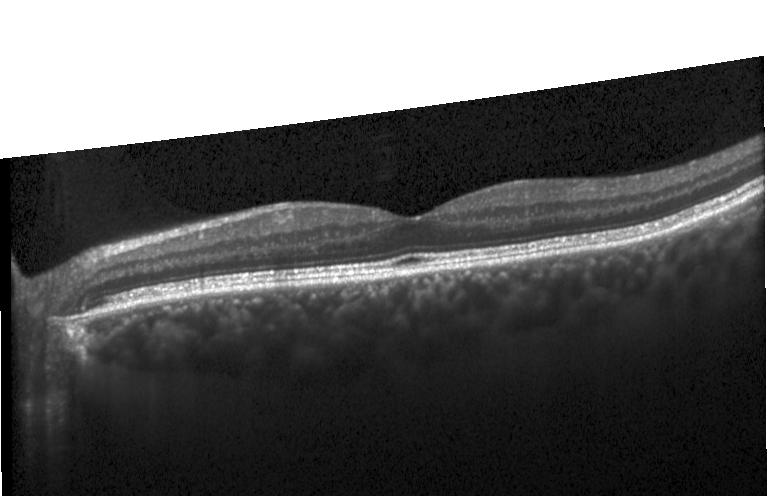

Optical coherence tomography scan — The scan shows neither choroidal neovascularization, diabetic macular edema, nor drusen.